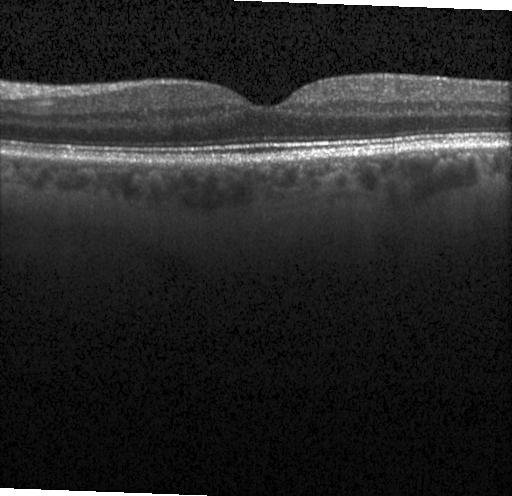 Diagnosis: no choroidal neovascularization, diabetic macular edema, or drusen.